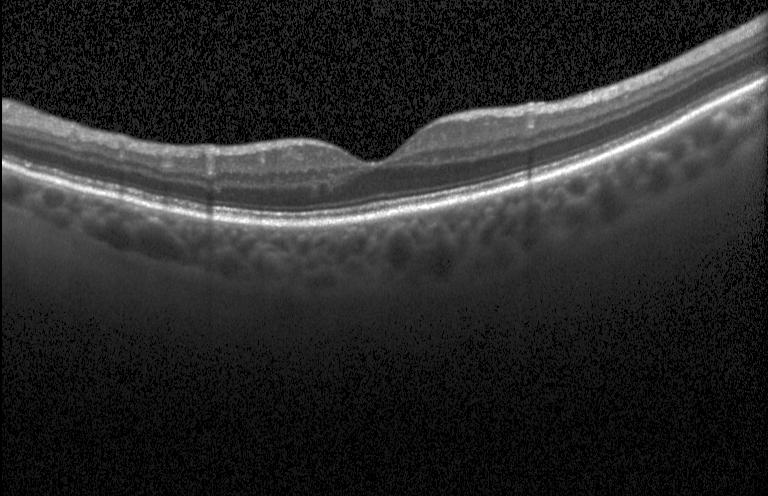 Retinal OCT B-scan — No choroidal neovascularization, no diabetic macular edema, and no drusen.